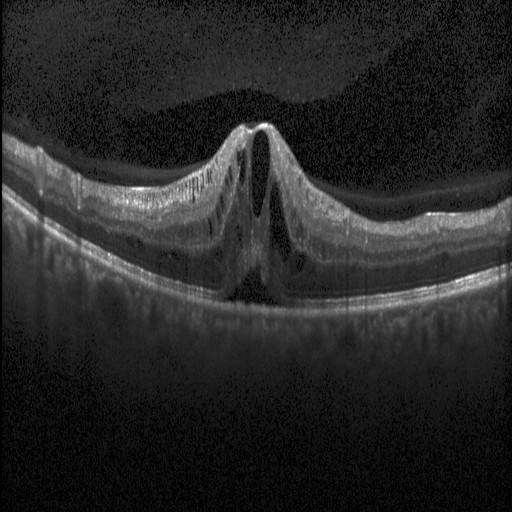 Assessment: DME.